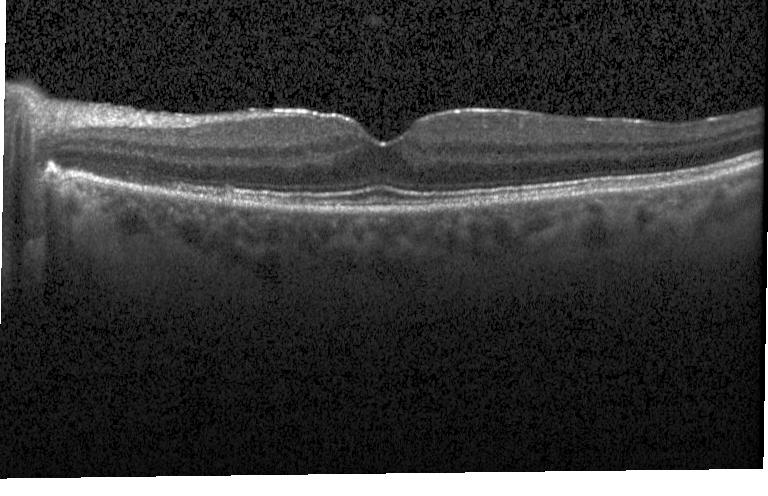 Spectral-domain OCT B-scan: no choroidal neovascularization, no diabetic macular edema, and no drusen.